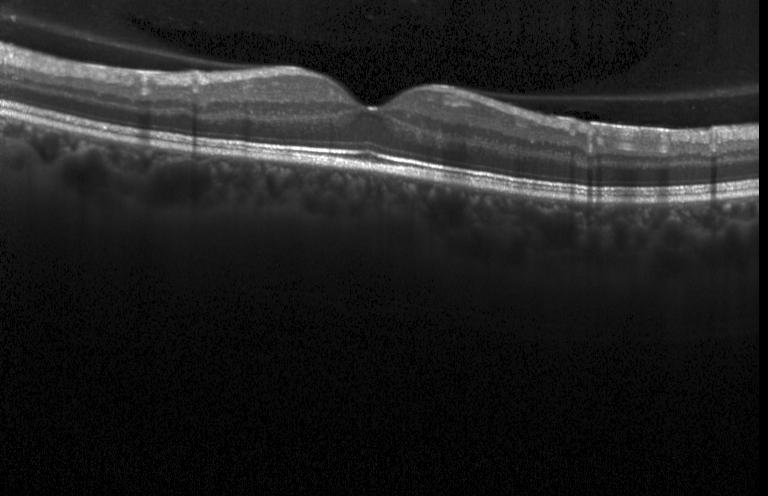
OCT line scan. Acquired on a Heidelberg Spectralis. Diagnosis: no choroidal neovascularization, diabetic macular edema, or drusen.